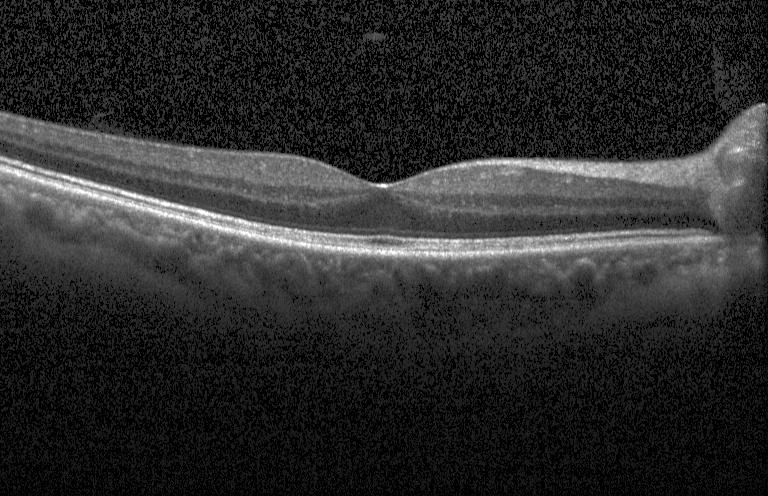 Heidelberg Spectralis OCT system, SD-OCT, fovea-centered, optical coherence tomography B-scan — No CNV, DME, or drusen.